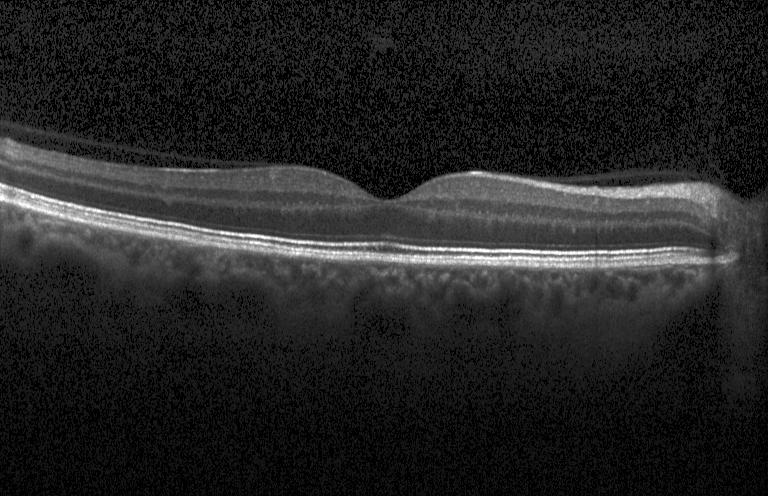

Dx: no CNV, no DME, and no drusen.